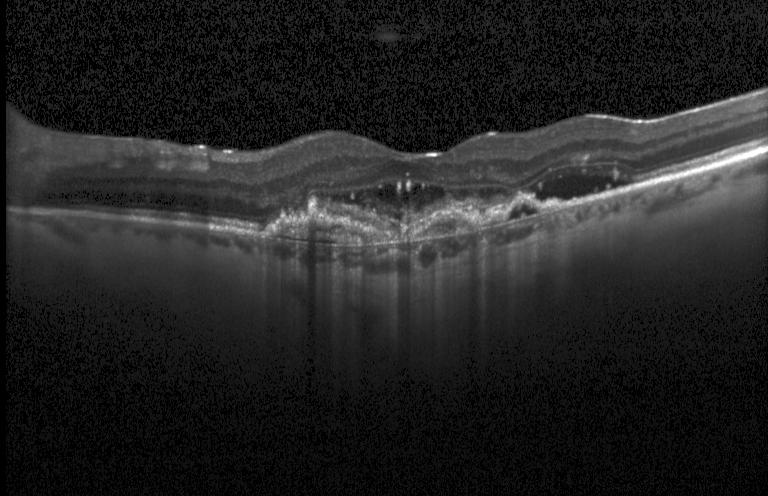
Optical coherence tomography scan
Macular OCT: choroidal neovascularization (CNV).